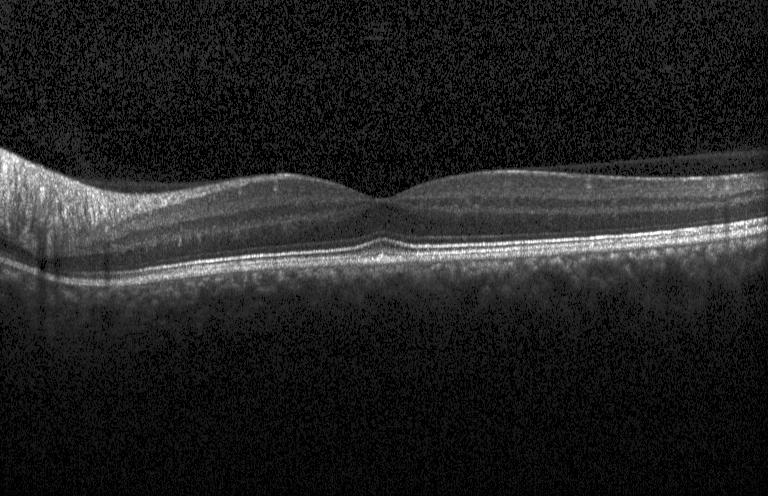 Optical coherence tomography scan. Dx: no choroidal neovascularization, diabetic macular edema, or drusen.